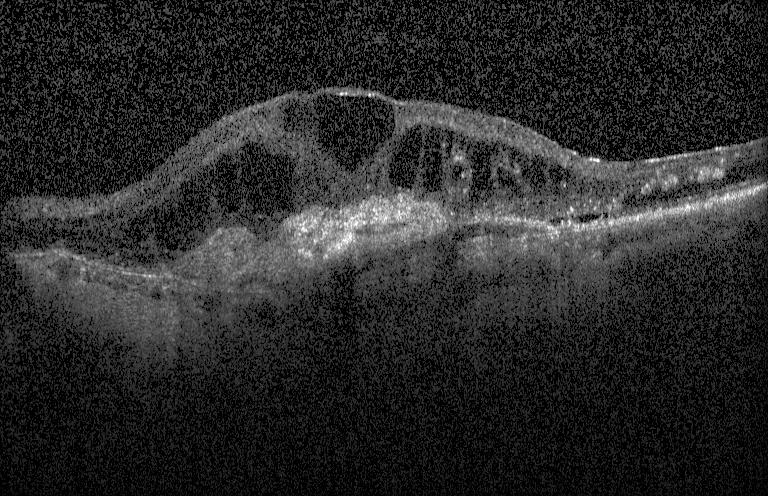
Macular scan · instrument: Heidelberg Spectralis · spectral-domain OCT · OCT B-scan. Diagnosis: a choroidal neovascular membrane.